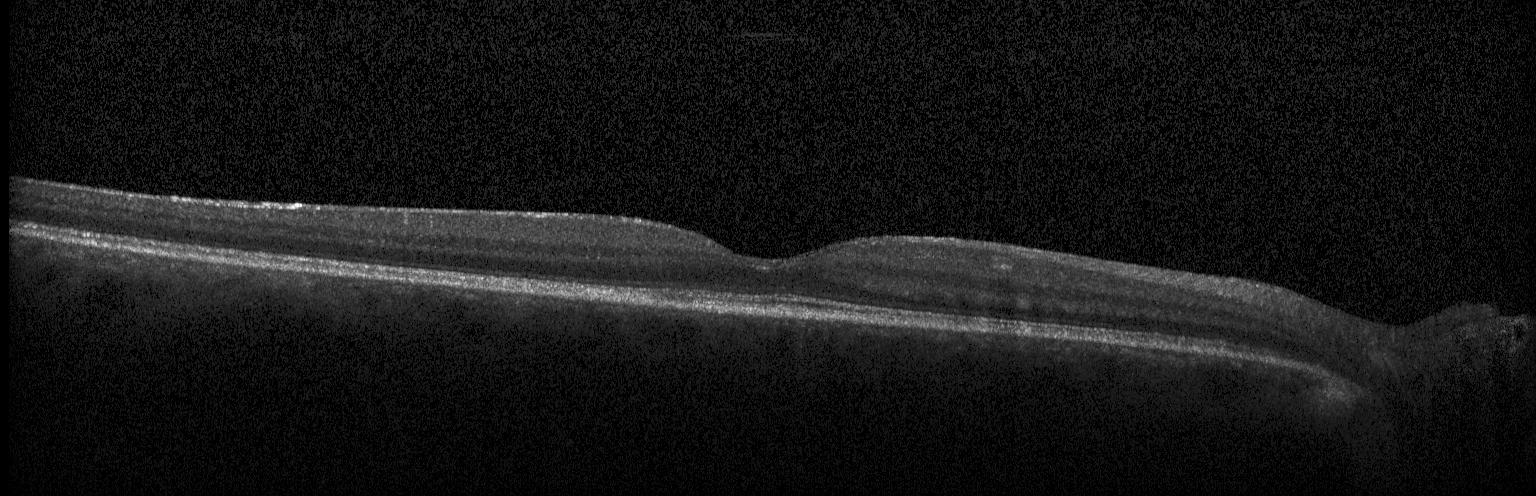
Spectral-domain OCT · Heidelberg Spectralis OCT system · retinal OCT B-scan.
The scan shows neither choroidal neovascularization, diabetic macular edema, nor drusen.